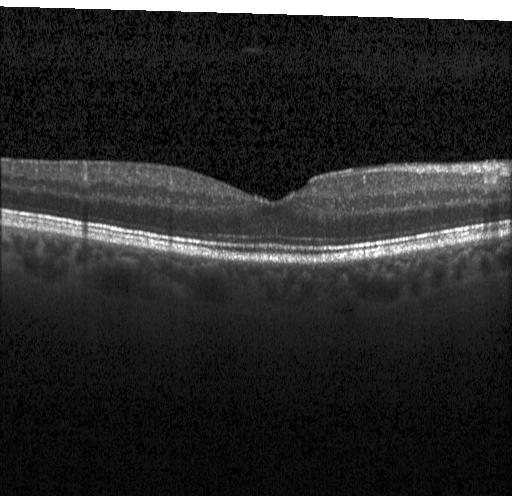
Optical coherence tomography B-scan · instrument: Heidelberg Spectralis · through the macula · SD-OCT
OCT finding: neither choroidal neovascularization, diabetic macular edema, nor drusen.